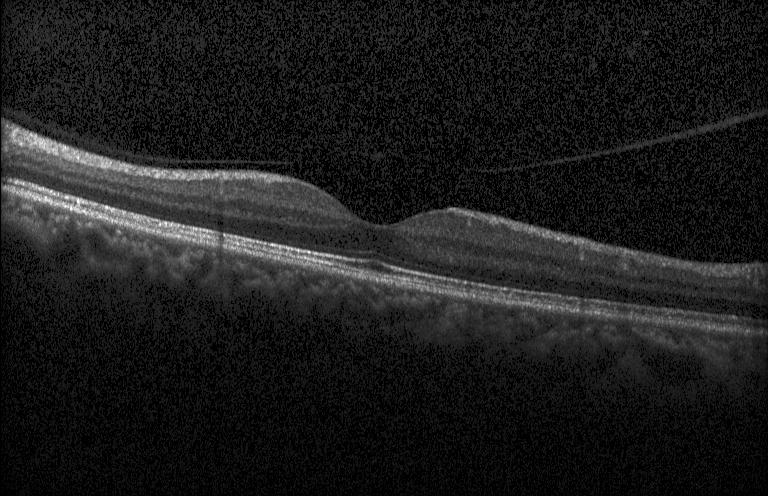
Dx: no evidence of choroidal neovascularization, diabetic macular edema, or drusen.